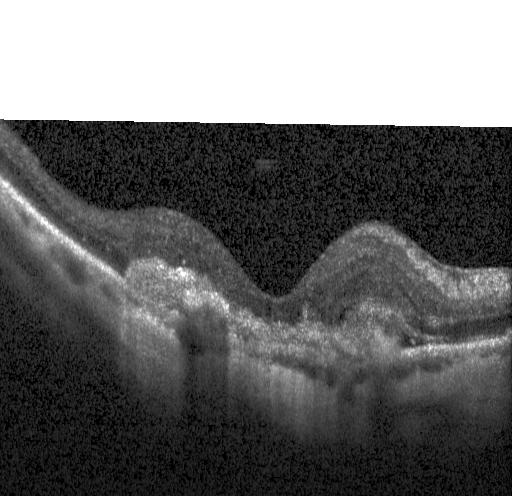
Optical coherence tomography scan. Horizontal scan through the fovea. Spectral-domain optical coherence tomography. Acquired on a Heidelberg Spectralis
The scan shows choroidal neovascularization.